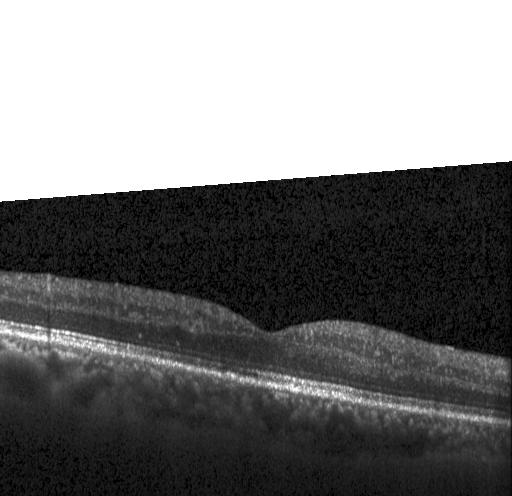
Macular scan; optical coherence tomography scan; spectral-domain OCT; instrument: Heidelberg Spectralis
Impression: no choroidal neovascularization, no diabetic macular edema, and no drusen.